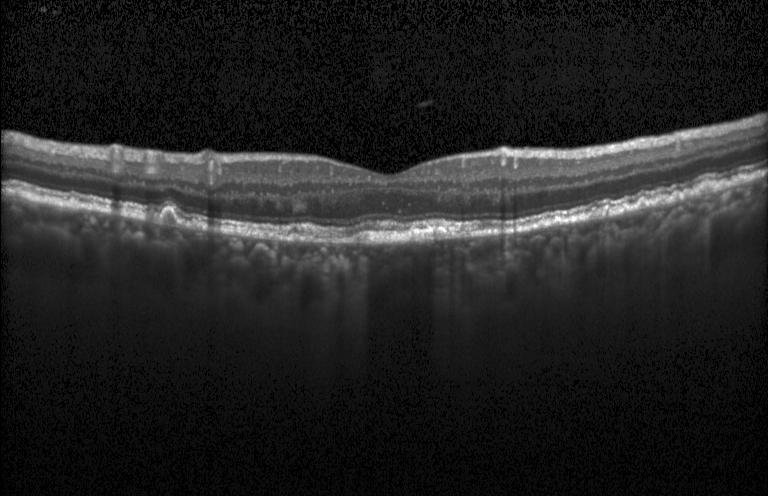 Macular scan; OCT B-scan.
Assessment: drusen.